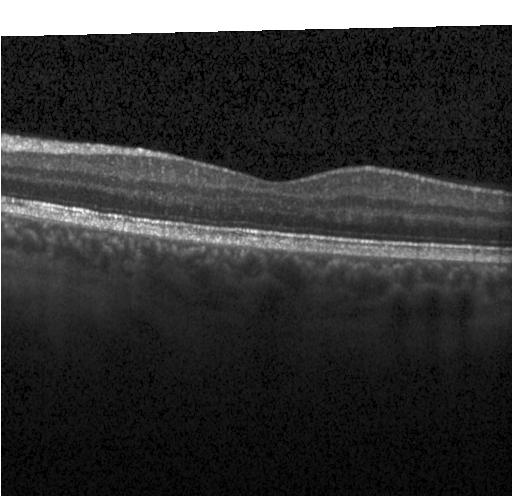 Heidelberg Spectralis OCT system, optical coherence tomography B-scan — OCT finding: neither CNV, DME, nor drusen.